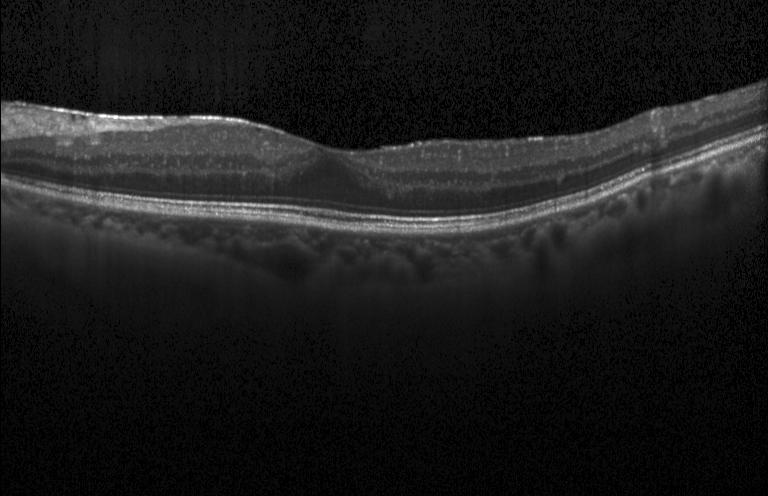 Impression: no evidence of choroidal neovascularization, diabetic macular edema, or drusen.